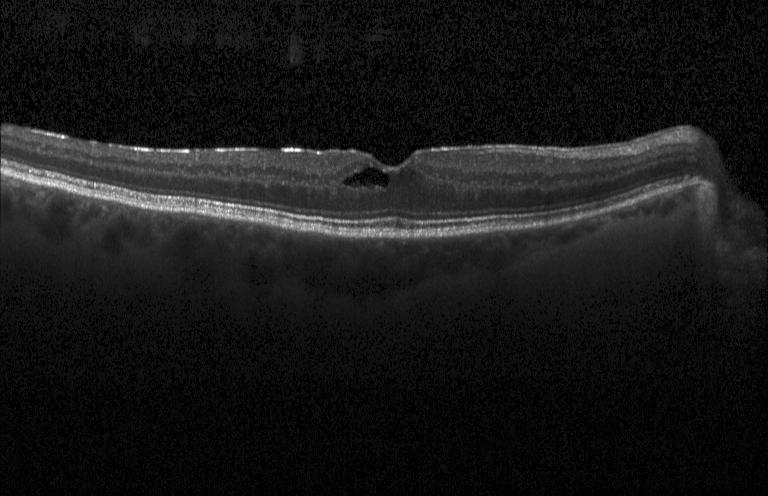

Instrument: Heidelberg Spectralis · macular scan · OCT line scan.
Finding: diabetic macular edema (DME).